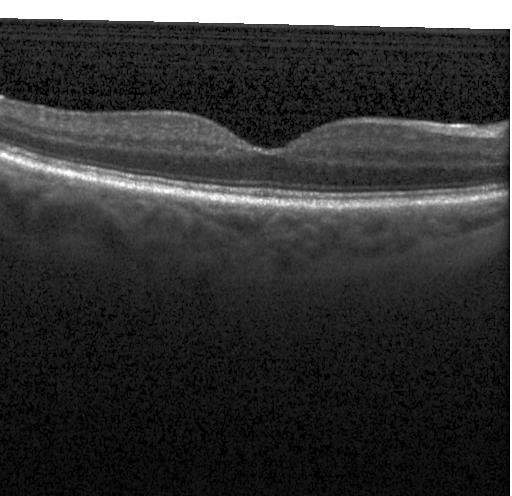 This B-scan demonstrates no choroidal neovascularization, no diabetic macular edema, and no drusen.